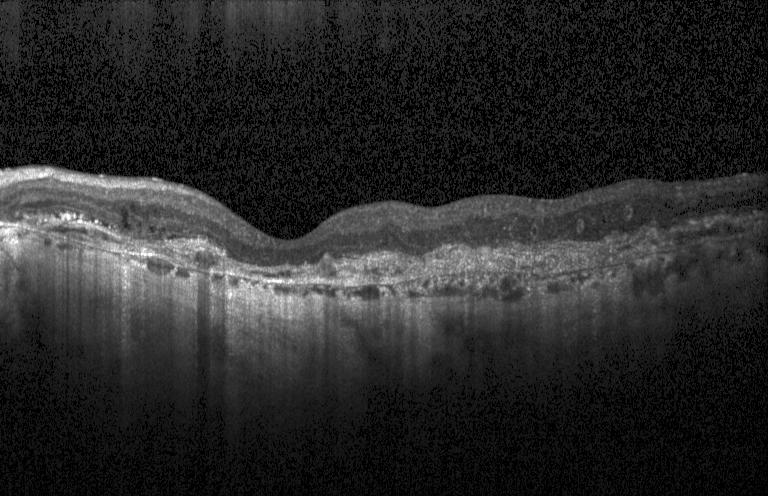 Optical coherence tomography B-scan, instrument: Heidelberg Spectralis, spectral-domain OCT, through the macula — Macular OCT: a choroidal neovascular membrane.